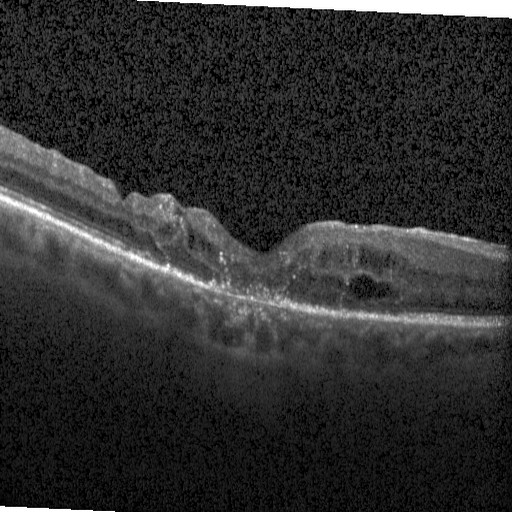

Dx: diabetic macular edema (DME).